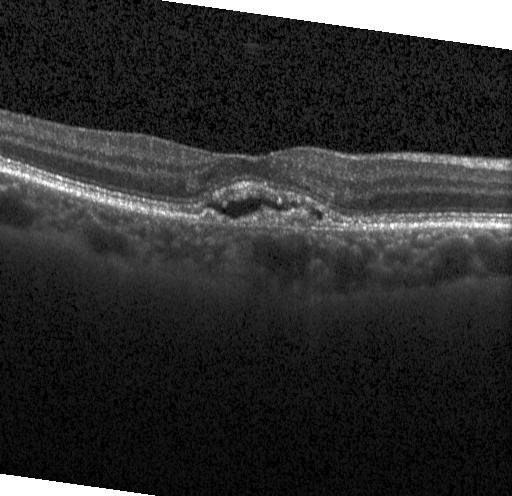
Optical coherence tomography scan
Diagnosis: a choroidal neovascular membrane.